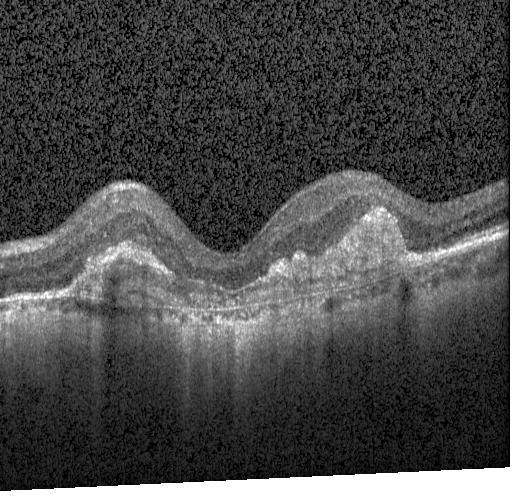
Impression: a choroidal neovascular membrane.